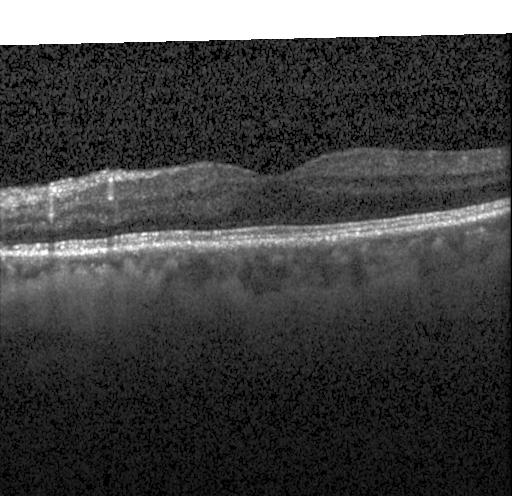 Acquired on a Heidelberg Spectralis · optical coherence tomography B-scan. OCT finding: no evidence of CNV, DME, or drusen.